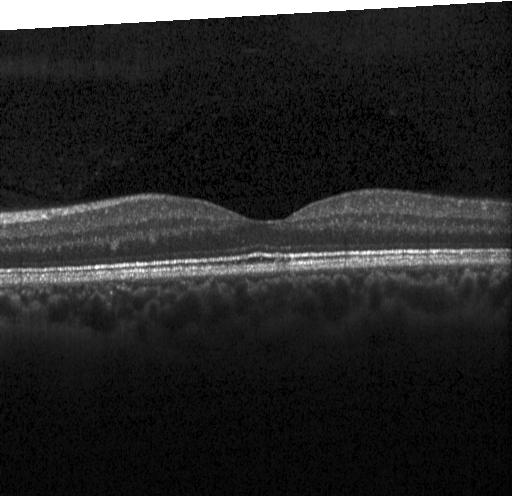
Retinal OCT cross-section. Macular OCT: no evidence of choroidal neovascularization, diabetic macular edema, or drusen.